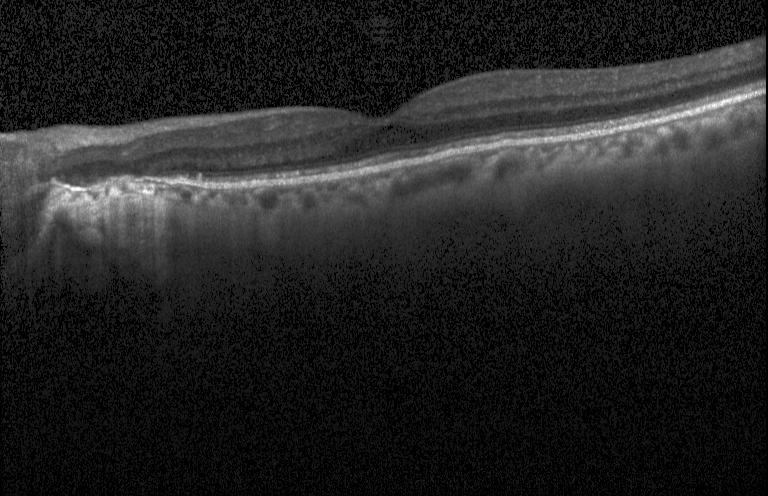 Instrument: Heidelberg Spectralis; retinal OCT B-scan; through the macula
The scan shows no choroidal neovascularization, no diabetic macular edema, and no drusen.